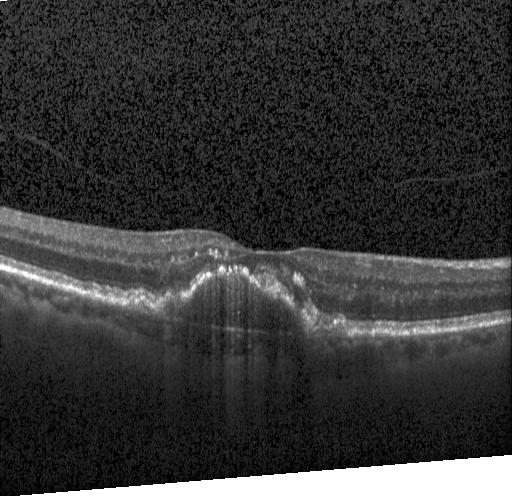
OCT B-scan showing CNV.